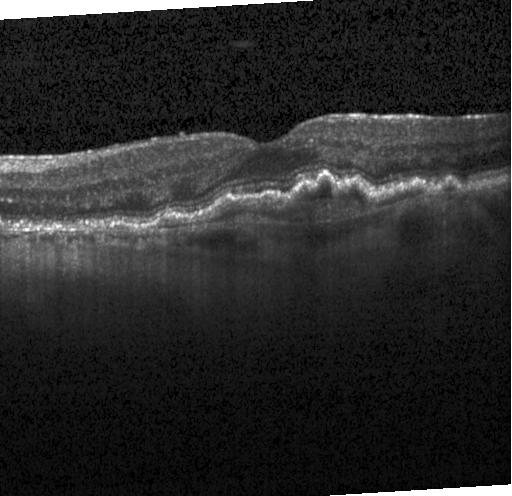 OCT line scan; instrument: Heidelberg Spectralis; horizontal scan through the fovea.
Dx: choroidal neovascularization (CNV).